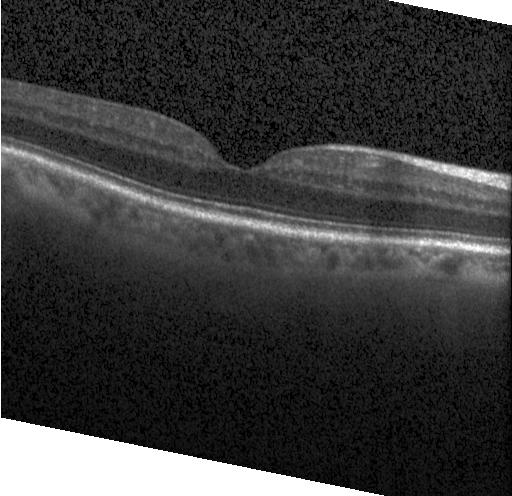
Horizontal scan through the fovea. OCT B-scan — Finding: no CNV, no DME, and no drusen.